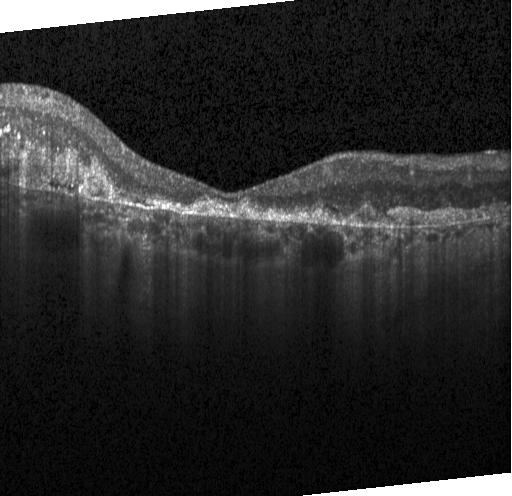
Fovea-centered; optical coherence tomography B-scan
Macular OCT: a choroidal neovascular membrane.